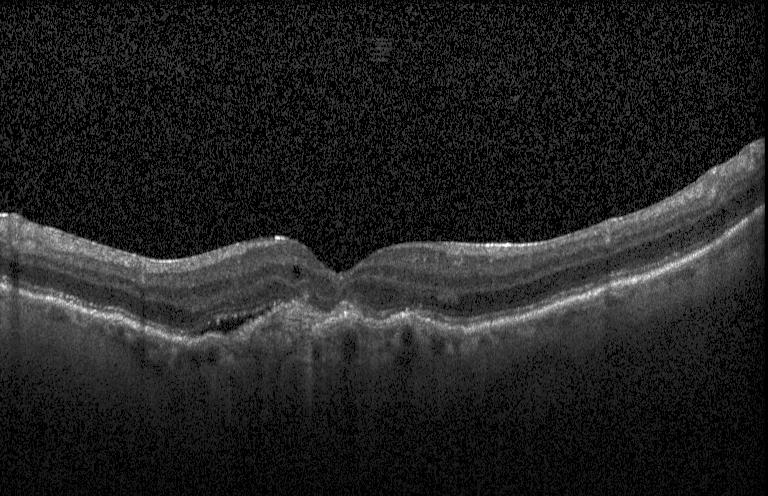 Diagnosis: choroidal neovascularization (CNV).